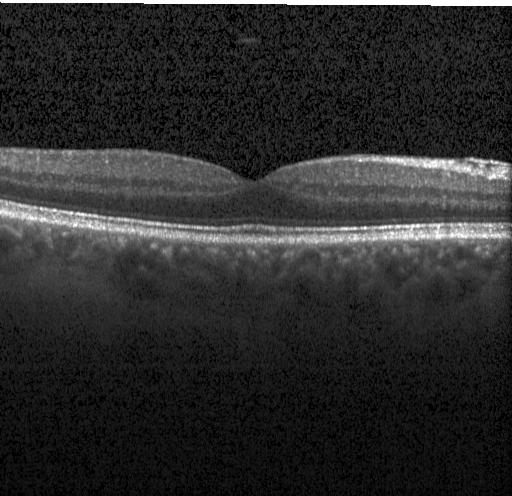
Macular OCT: no choroidal neovascularization, no diabetic macular edema, and no drusen.